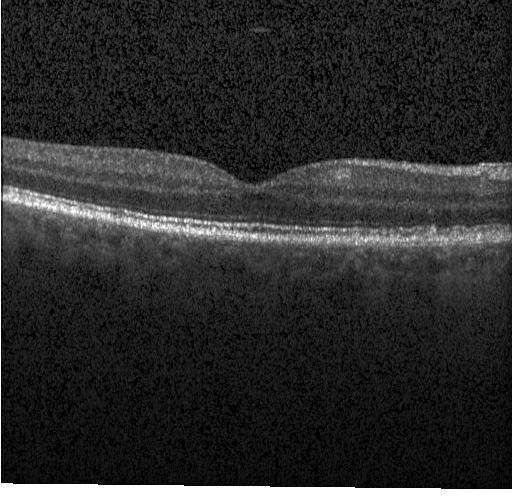 Diagnosis: multiple drusen.